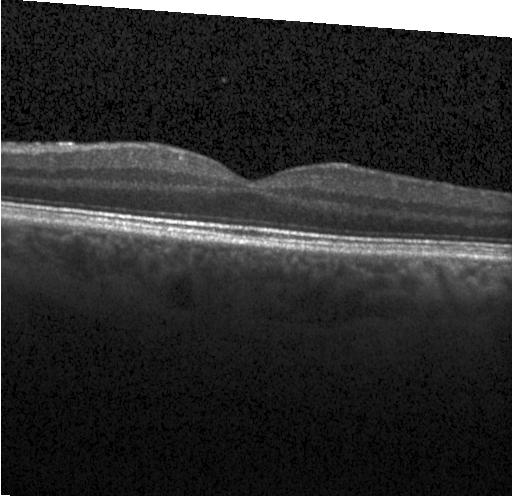 Finding: neither CNV, DME, nor drusen.